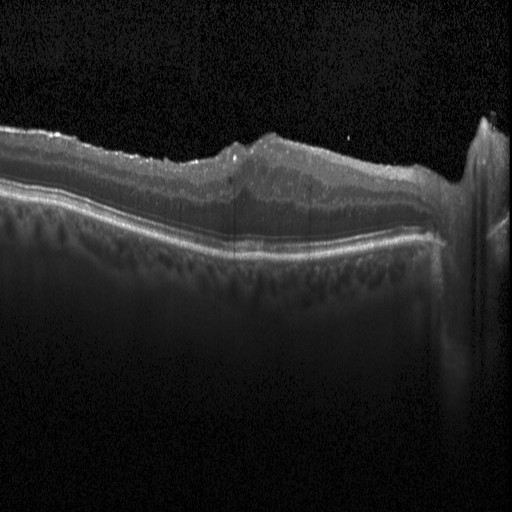 OCT finding: diabetic macular edema (DME).